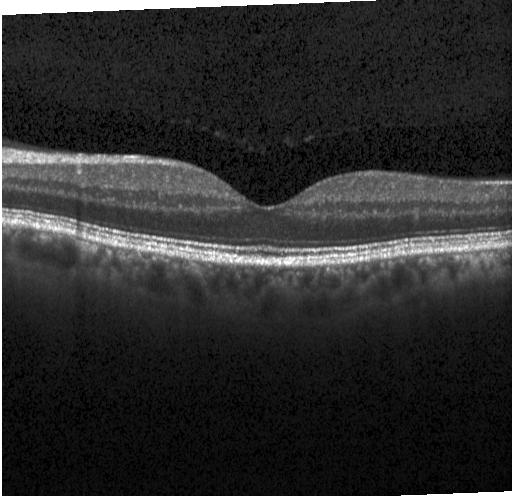
OCT B-scan. Assessment: no choroidal neovascularization, diabetic macular edema, or drusen.